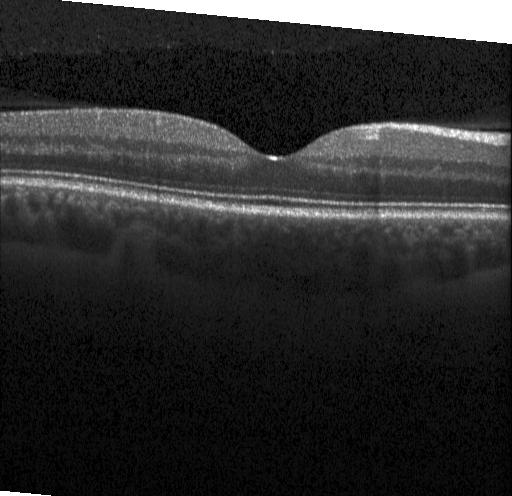
Through the macula; OCT B-scan; SD-OCT
Impression: no CNV, DME, or drusen.